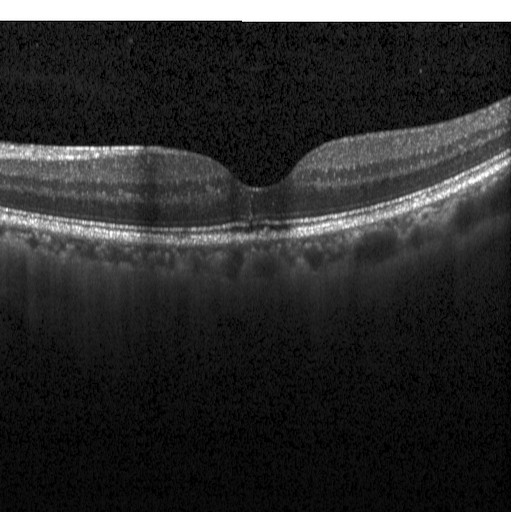 Spectral-domain optical coherence tomography. Horizontal scan through the fovea. OCT B-scan. Acquired on a Heidelberg Spectralis — Dx: diabetic macular edema.